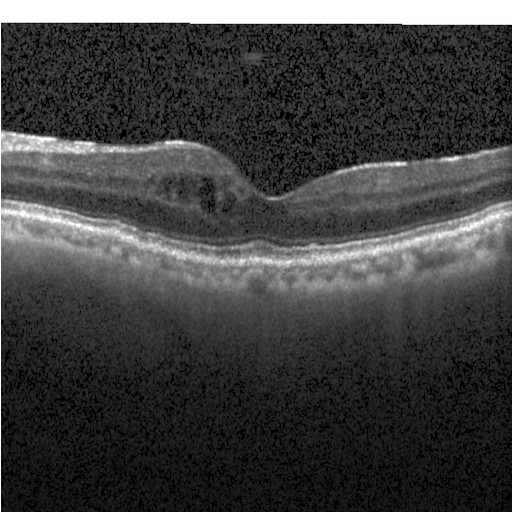
Retinal OCT cross-section showing DME.